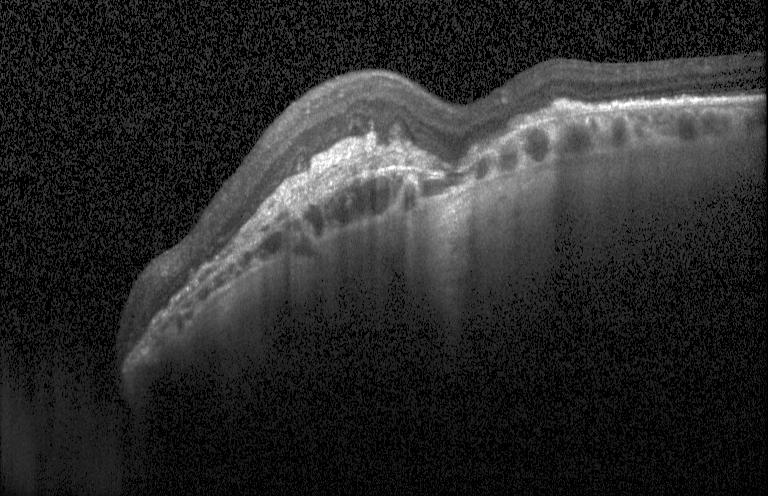

Optical coherence tomography scan
Choroidal neovascularization.